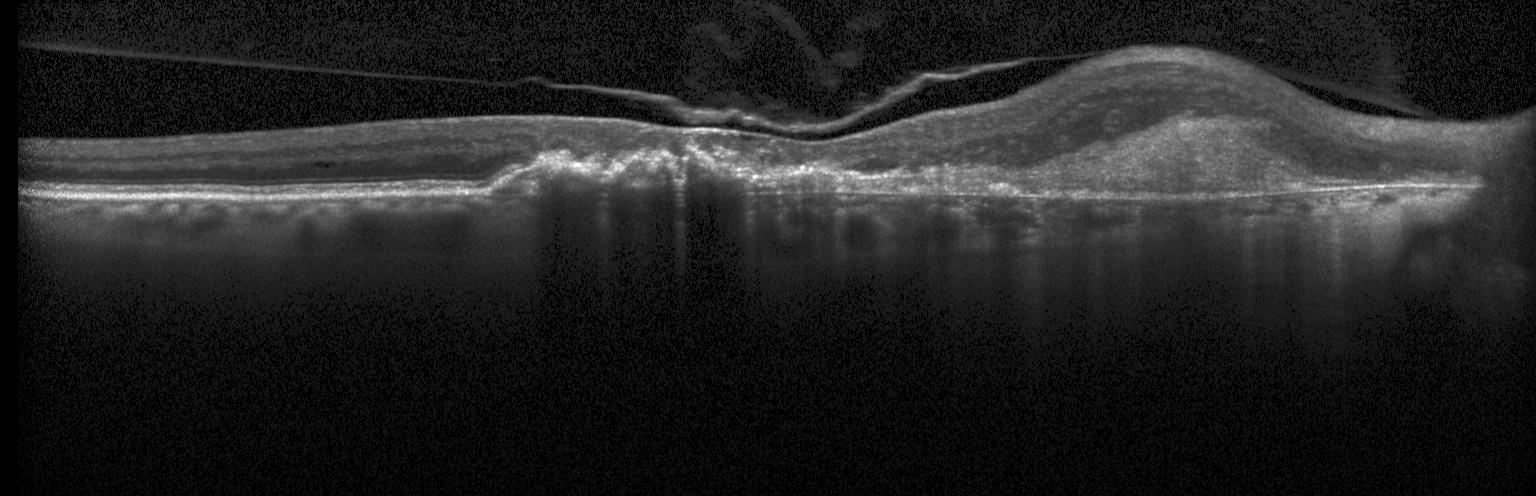

Macular OCT: a choroidal neovascular membrane.